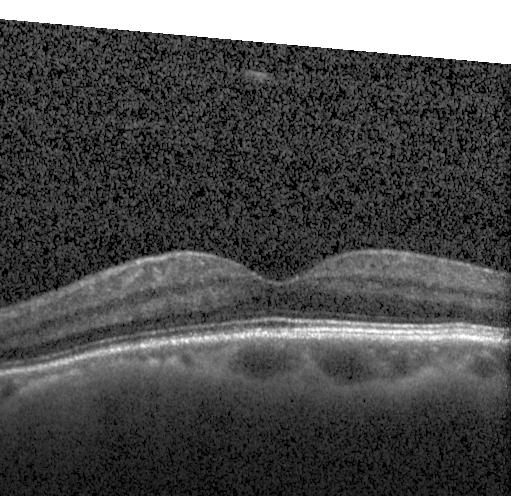 Macular OCT demonstrating neither CNV, DME, nor drusen.